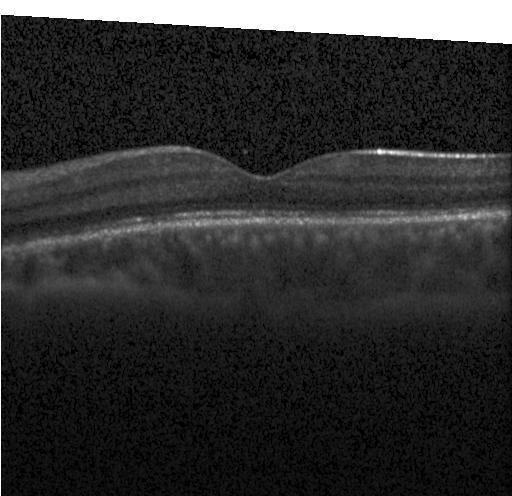
Optical coherence tomography scan, instrument: Heidelberg Spectralis
This B-scan demonstrates no choroidal neovascularization, no diabetic macular edema, and no drusen.